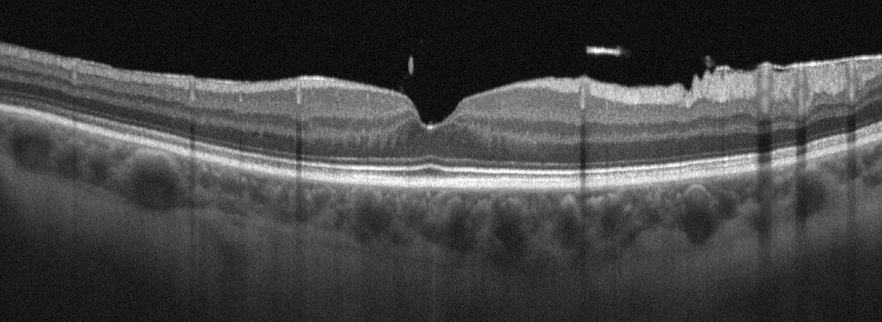

Optovue Avanti RTVue XR, retinal OCT B-scan, left eye. Finding: epiretinal membrane.